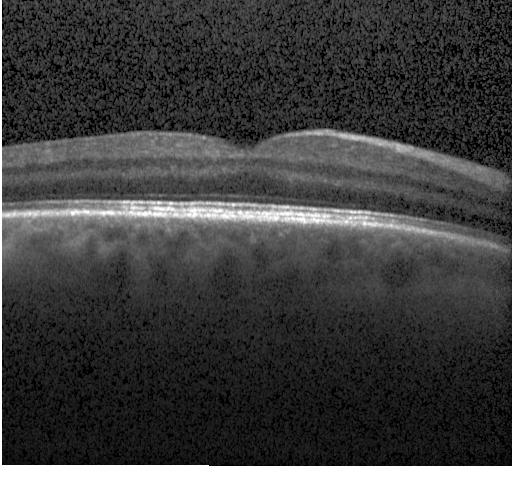 Diagnosis: no evidence of choroidal neovascularization, diabetic macular edema, or drusen.